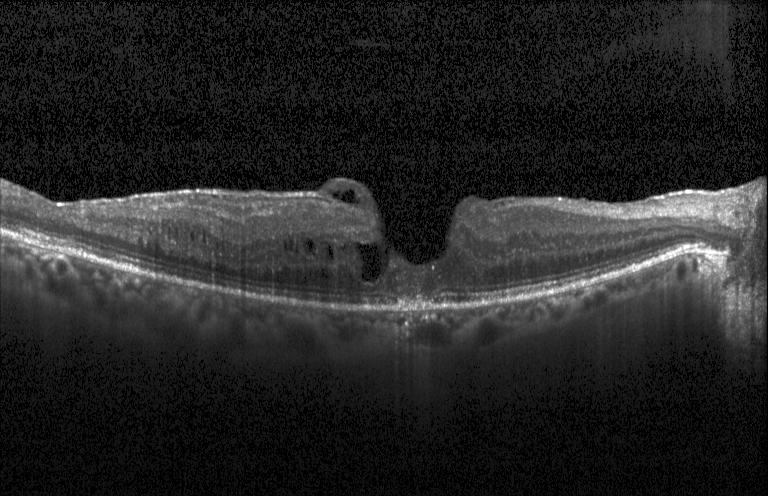 Macular OCT demonstrating diabetic macular edema.